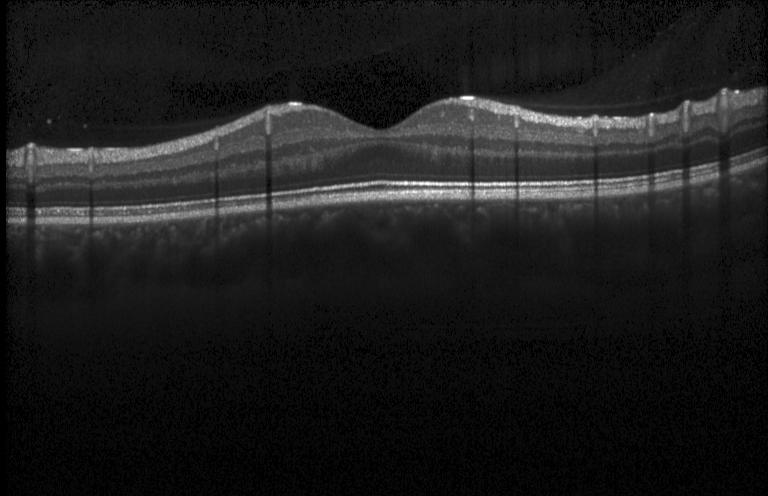 The scan shows neither choroidal neovascularization, diabetic macular edema, nor drusen.